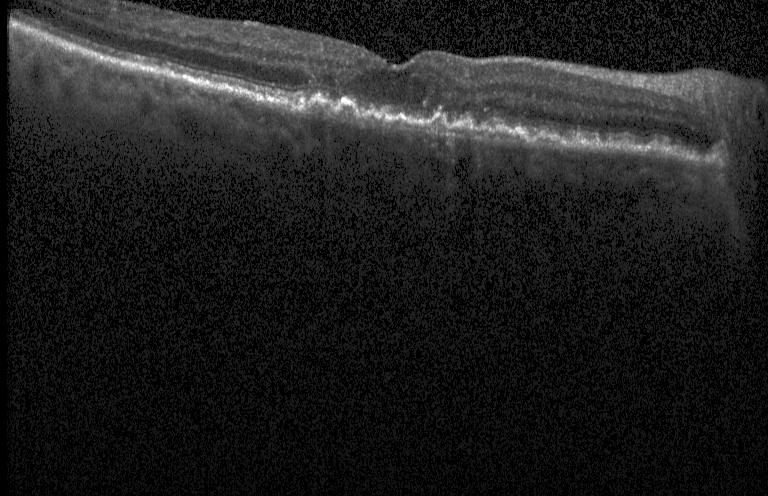
This B-scan demonstrates sub-RPE drusenoid deposits.